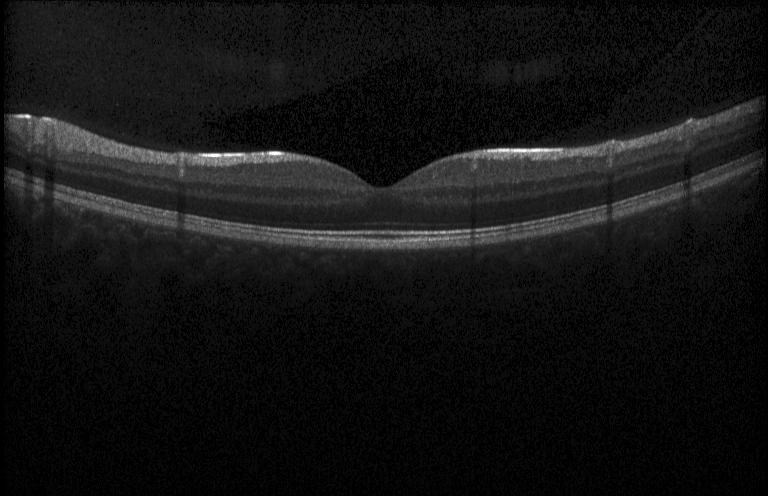

OCT line scan — Diagnosis: neither choroidal neovascularization, diabetic macular edema, nor drusen.